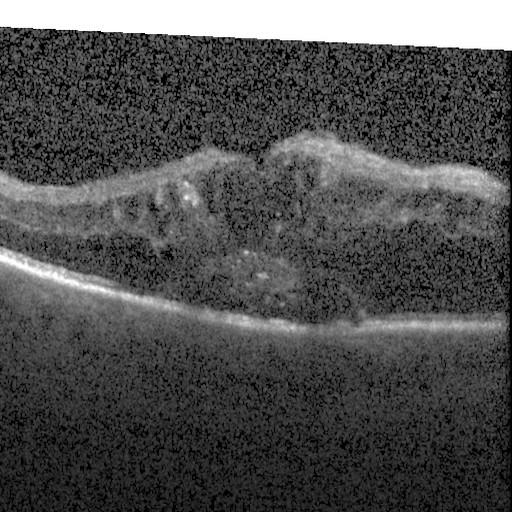 The scan shows diabetic macular edema.